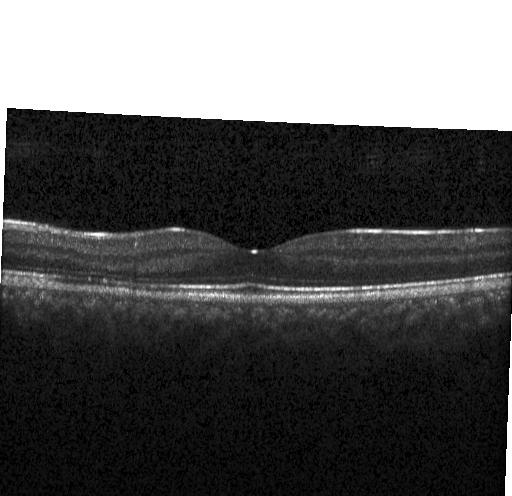
Retinal OCT cross-section.
OCT finding: no evidence of choroidal neovascularization, diabetic macular edema, or drusen.